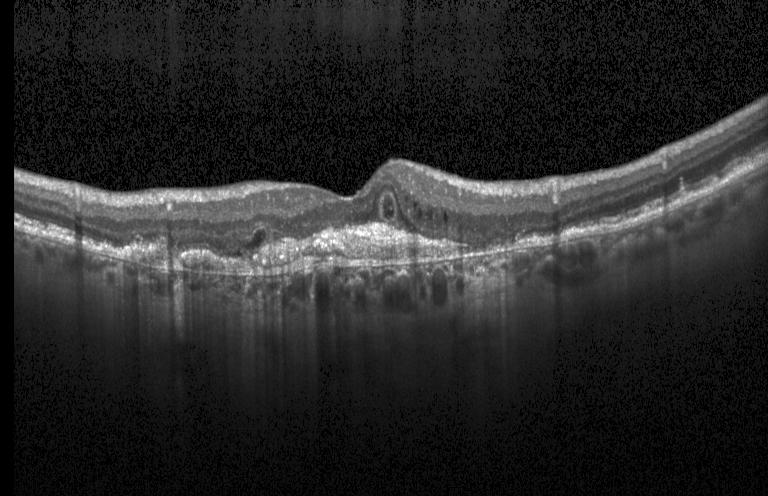
Retinal OCT B-scan — The scan shows choroidal neovascularization (CNV).